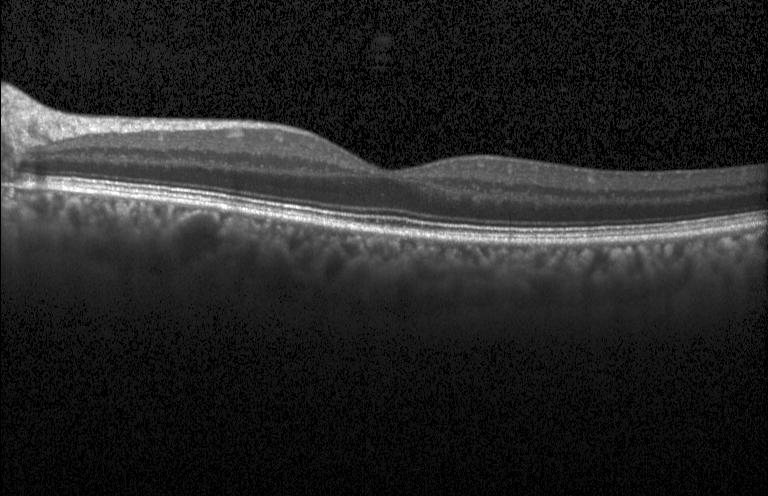 Spectral-domain optical coherence tomography; Heidelberg Spectralis OCT system; optical coherence tomography B-scan; through the macula. Assessment: neither choroidal neovascularization, diabetic macular edema, nor drusen.